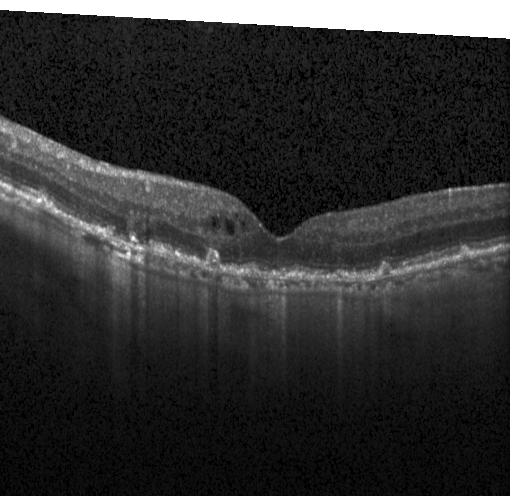
Retinal OCT cross-section — Macular OCT: a choroidal neovascular membrane.